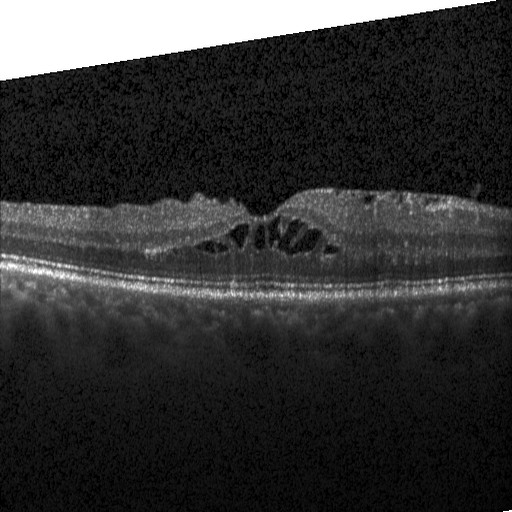
Optical coherence tomography scan
The scan shows diabetic macular edema.